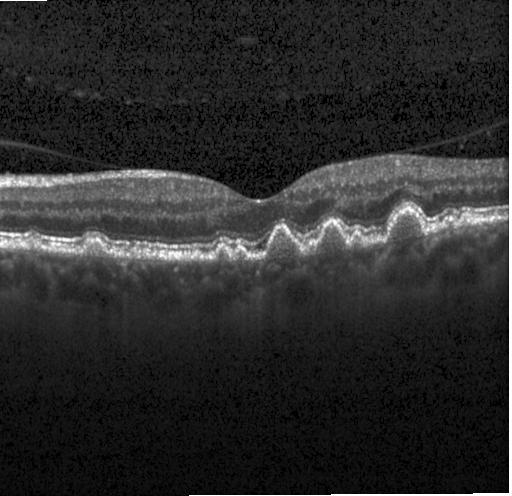 OCT B-scan.
Diagnosis: sub-RPE drusenoid deposits.